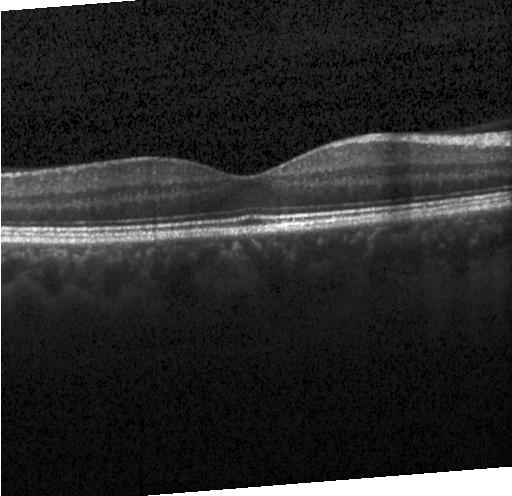 Spectral-domain optical coherence tomography; acquired on a Heidelberg Spectralis; retinal OCT cross-section; through the macula
Macular OCT: no CNV, no DME, and no drusen.